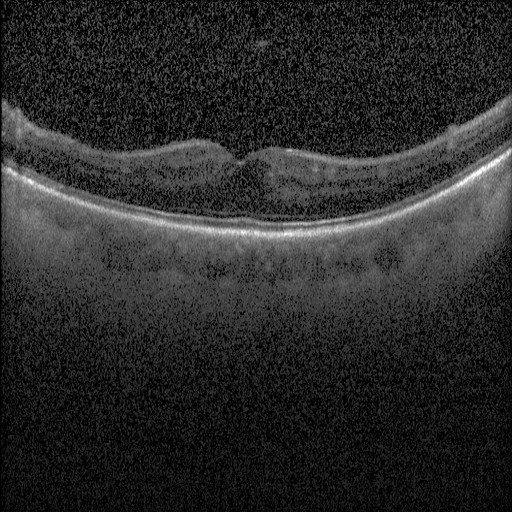
OCT B-scan — Macular OCT: diabetic macular edema.